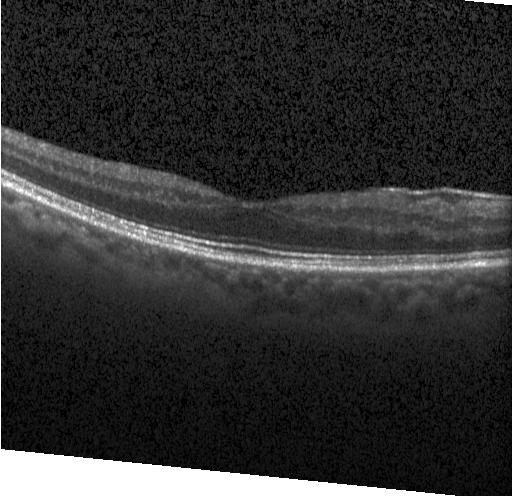
Heidelberg Spectralis OCT system, OCT B-scan, spectral-domain OCT. Impression: no choroidal neovascularization, no diabetic macular edema, and no drusen.